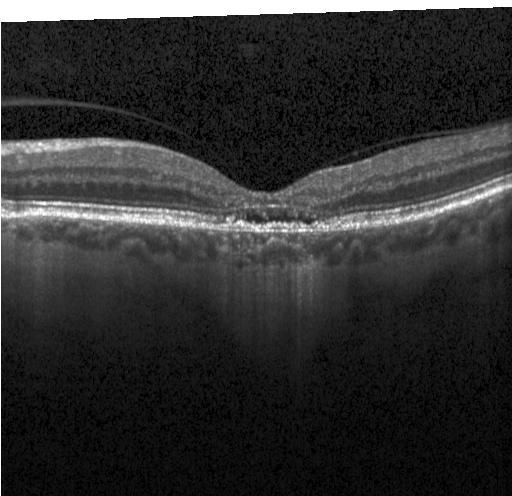

Retinal OCT B-scan — Finding: a choroidal neovascular membrane.